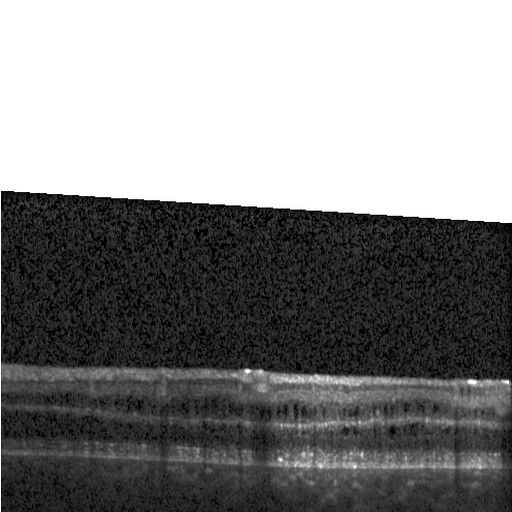

Spectral-domain OCT. Fovea-centered. Heidelberg Spectralis. OCT line scan.
Dx: DME.